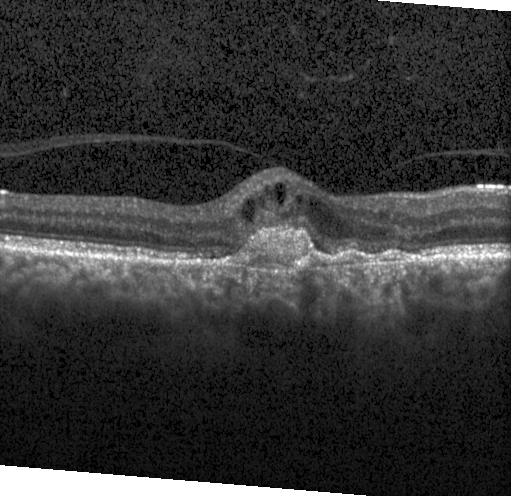 Fovea-centered; retinal OCT B-scan.
Dx: choroidal neovascularization (CNV).